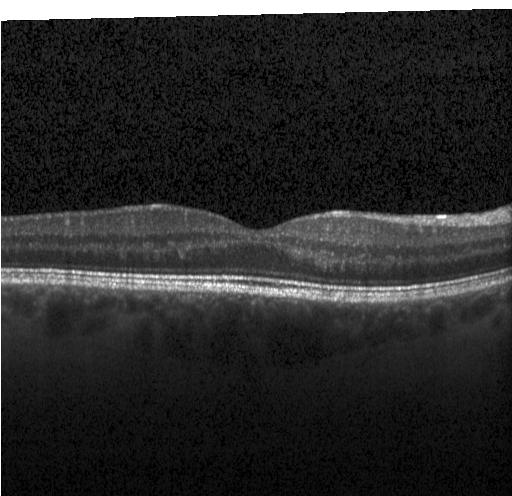 Finding: neither choroidal neovascularization, diabetic macular edema, nor drusen.